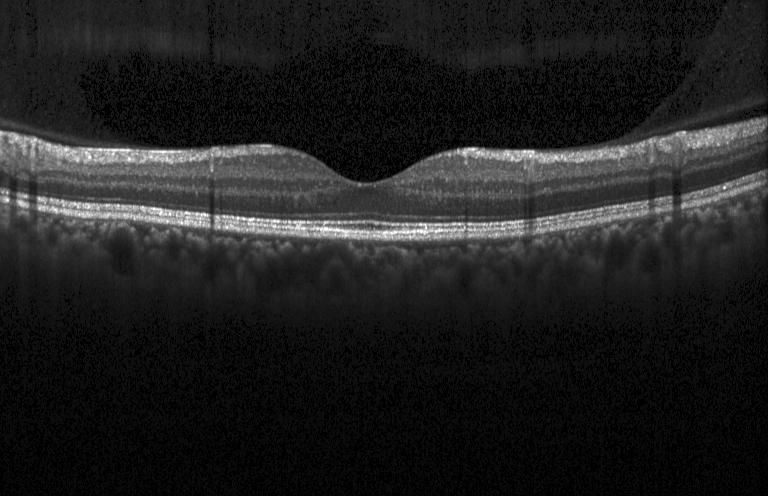

OCT B-scan · instrument: Heidelberg Spectralis · horizontal scan through the fovea.
Neither CNV, DME, nor drusen.